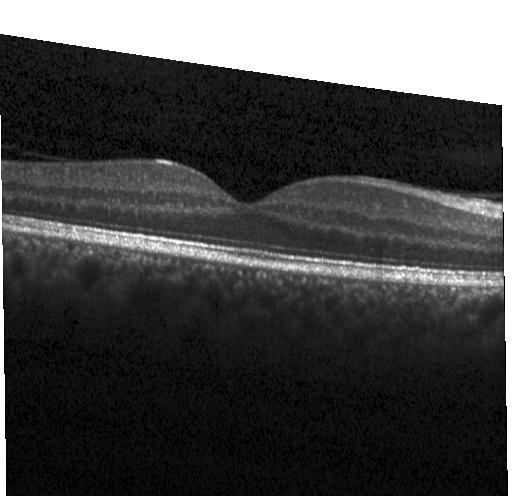
No choroidal neovascularization, no diabetic macular edema, and no drusen.